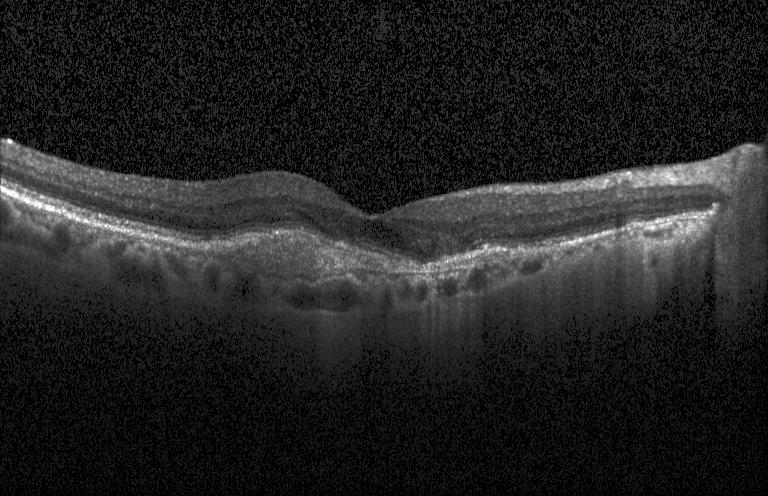
Optical coherence tomography scan, instrument: Heidelberg Spectralis, through the macula — Finding: choroidal neovascularization (CNV).